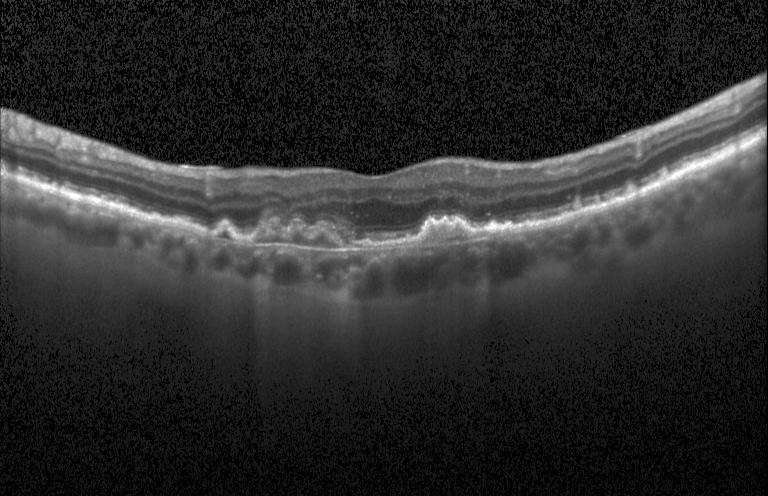
Spectral-domain optical coherence tomography. Optical coherence tomography B-scan. Fovea-centered. Acquired on a Heidelberg Spectralis
This B-scan demonstrates drusen.